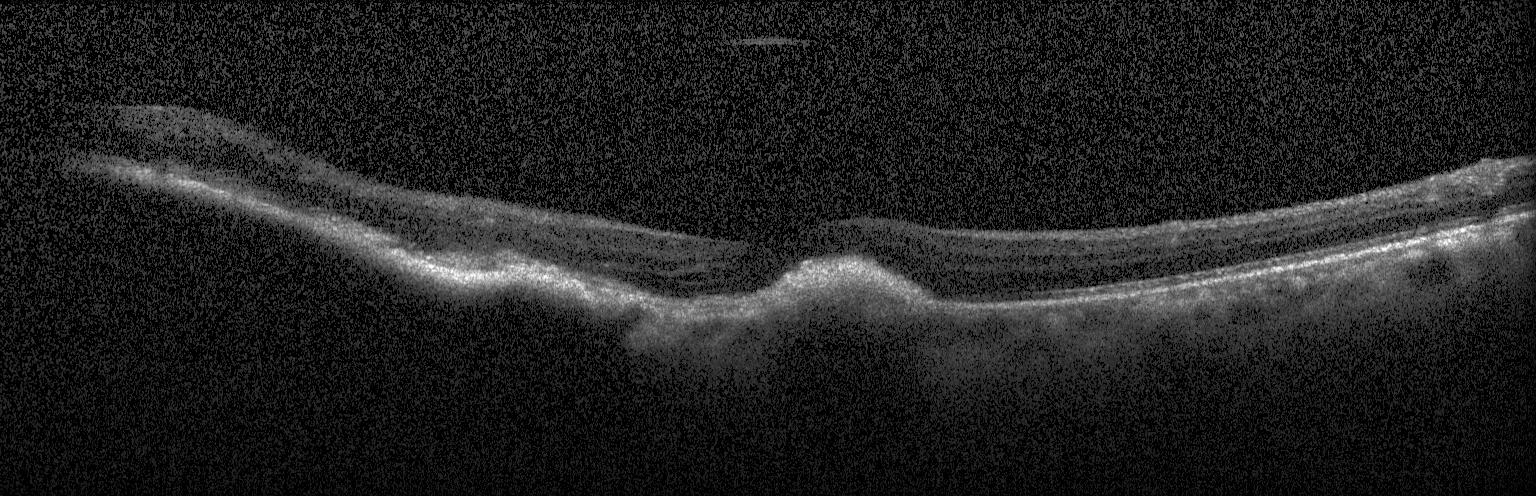 Finding: a choroidal neovascular membrane.